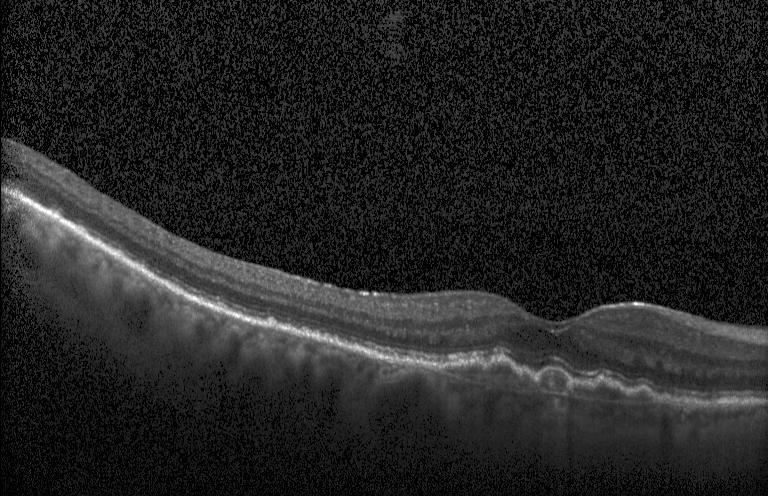
OCT line scan; acquired on a Heidelberg Spectralis; centered on the fovea — OCT finding: CNV.